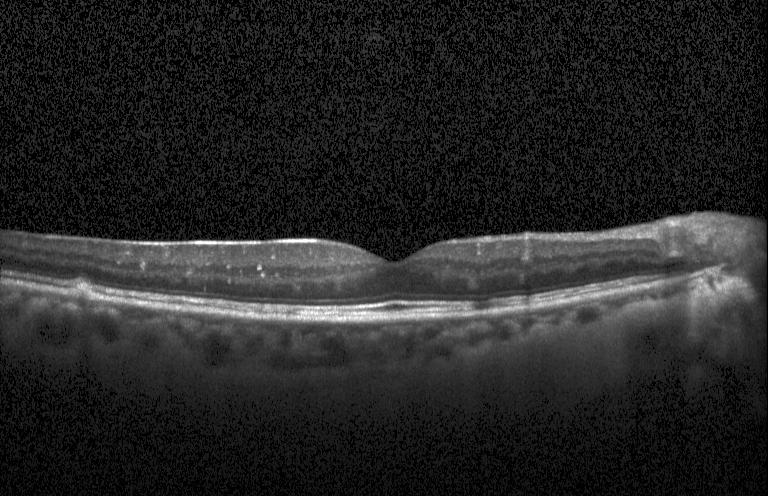 SD-OCT, optical coherence tomography B-scan
Finding: no evidence of CNV, DME, or drusen.